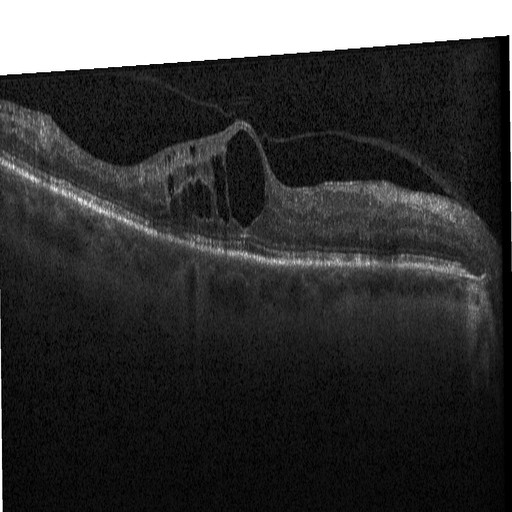 Finding: diabetic macular edema.